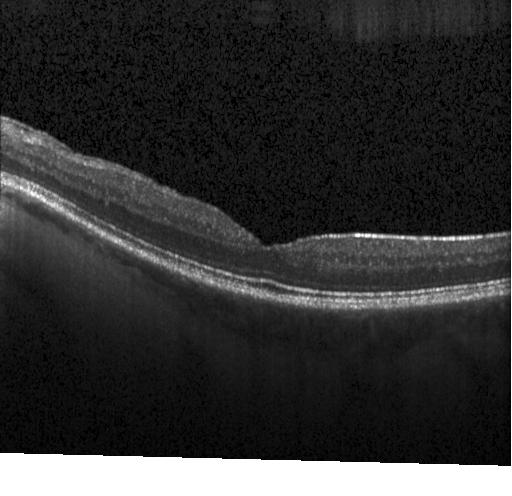

Finding: no CNV, DME, or drusen.